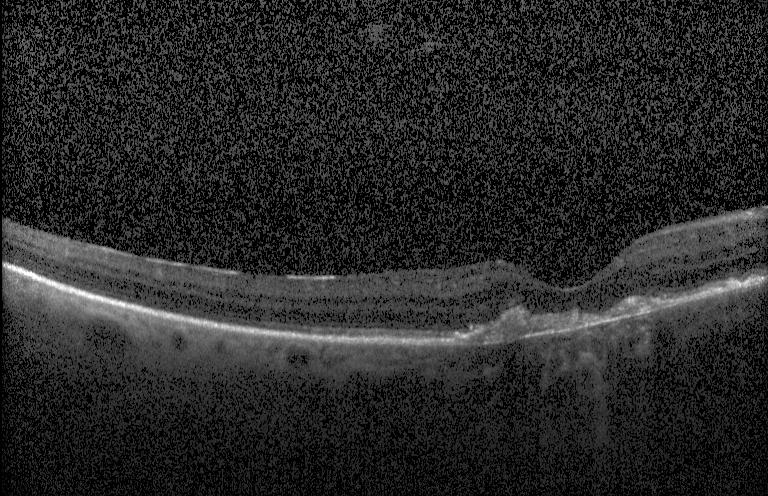 Spectral-domain optical coherence tomography. Instrument: Heidelberg Spectralis. Retinal OCT B-scan
Diagnosis: a choroidal neovascular membrane.